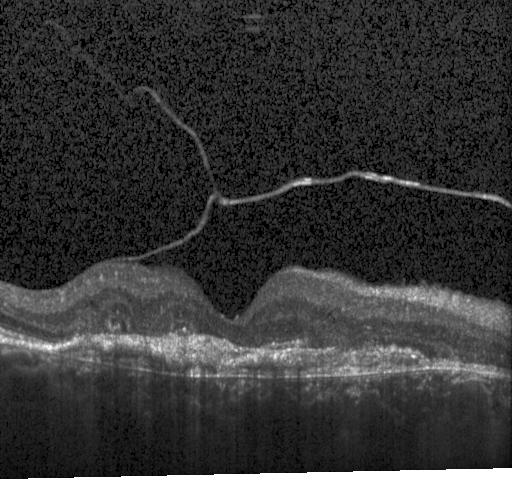
OCT B-scan · Heidelberg Spectralis · SD-OCT · macular scan — Finding: a choroidal neovascular membrane.